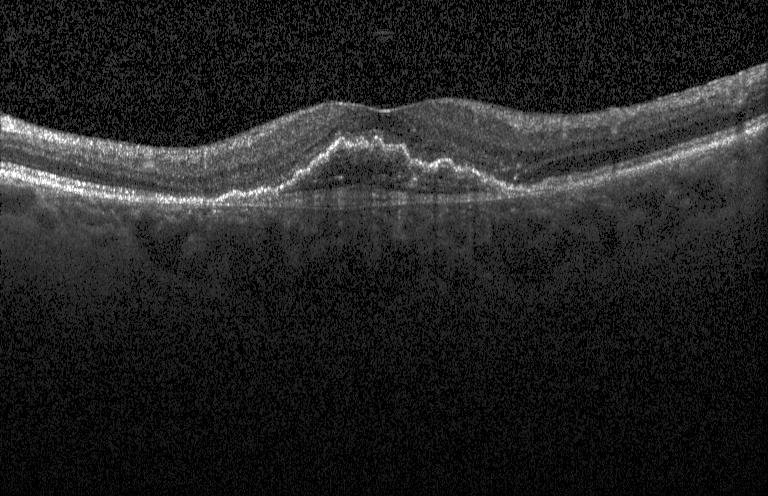 Optical coherence tomography scan · centered on the fovea
Macular OCT: CNV.